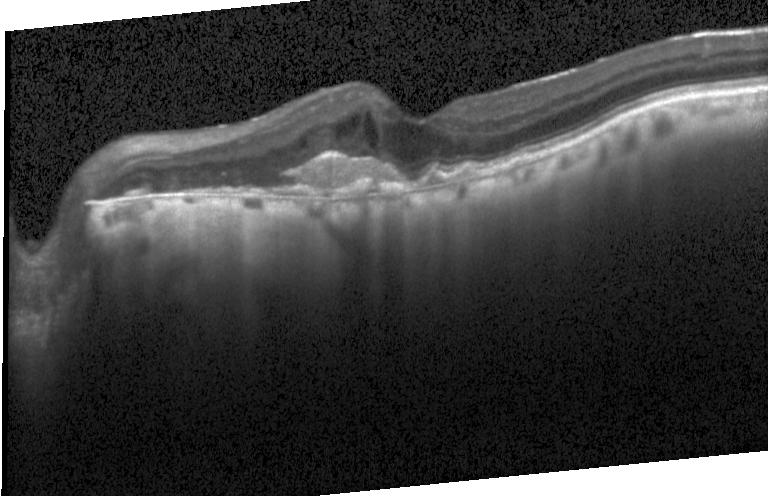 Spectral-domain optical coherence tomography; horizontal scan through the fovea; optical coherence tomography B-scan; Heidelberg Spectralis
Macular OCT: choroidal neovascularization (CNV).